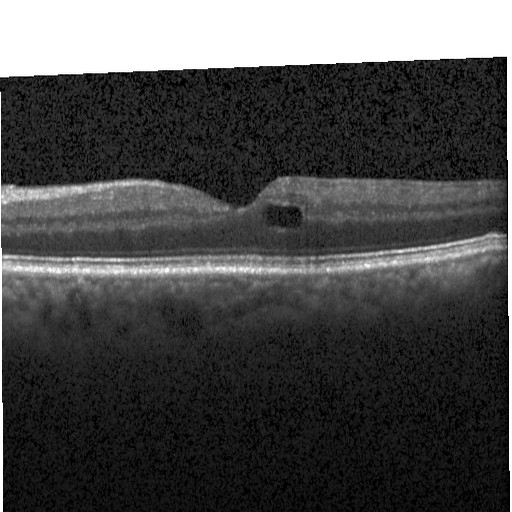
The scan shows diabetic macular edema.